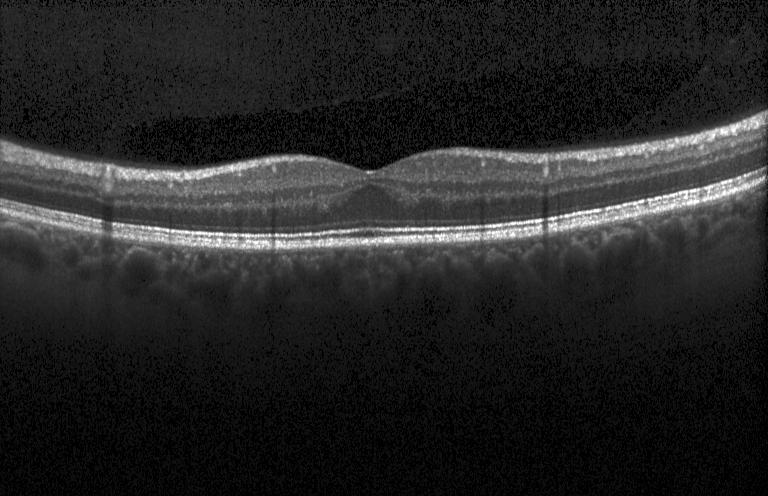

Retinal OCT B-scan — Diagnosis: no CNV, DME, or drusen.